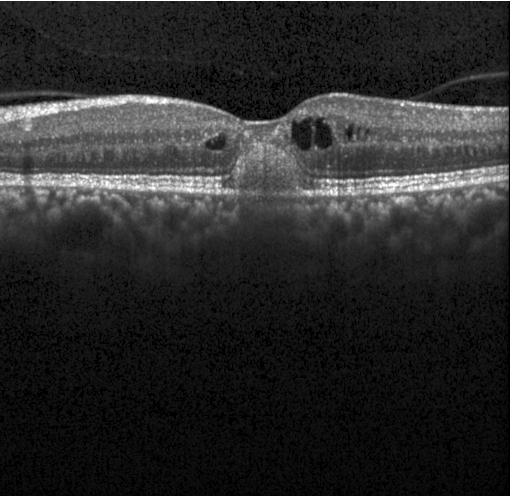 Retinal OCT cross-section; Heidelberg Spectralis OCT system; spectral-domain optical coherence tomography — Dx: a choroidal neovascular membrane.